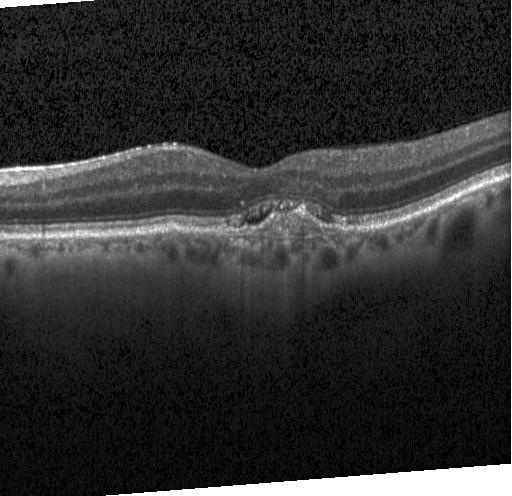 Retinal OCT cross-section
Impression: CNV.